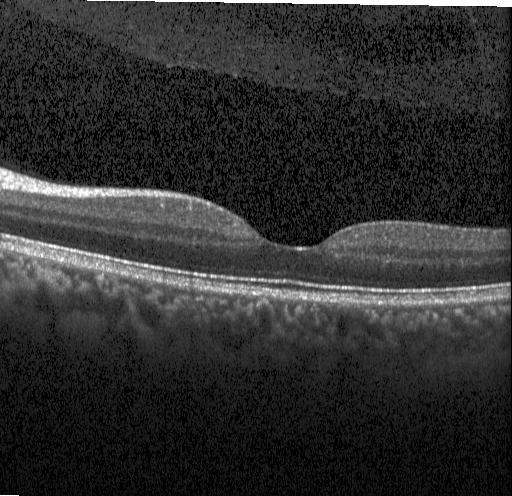 Diagnosis: neither choroidal neovascularization, diabetic macular edema, nor drusen.